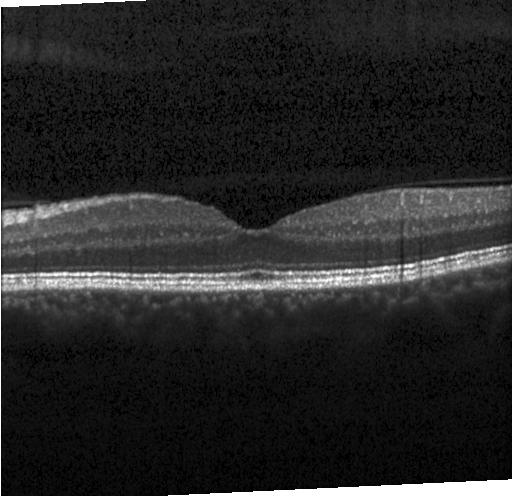
Macular scan. Spectral-domain optical coherence tomography. OCT B-scan. Diagnosis: neither CNV, DME, nor drusen.